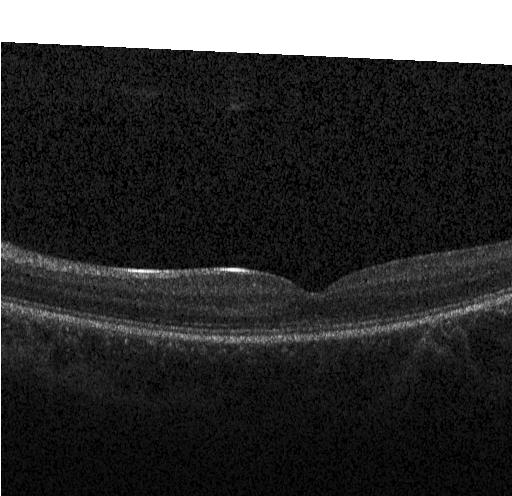 OCT finding: no CNV, no DME, and no drusen.